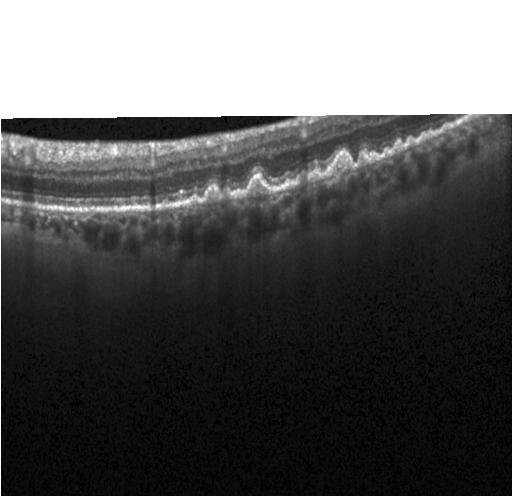 Optical coherence tomography B-scan — Diagnosis: drusen.